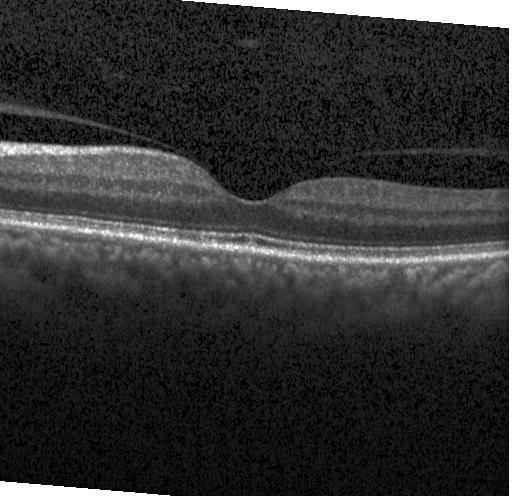
Heidelberg Spectralis, through the macula, OCT line scan. Macular OCT: neither choroidal neovascularization, diabetic macular edema, nor drusen.